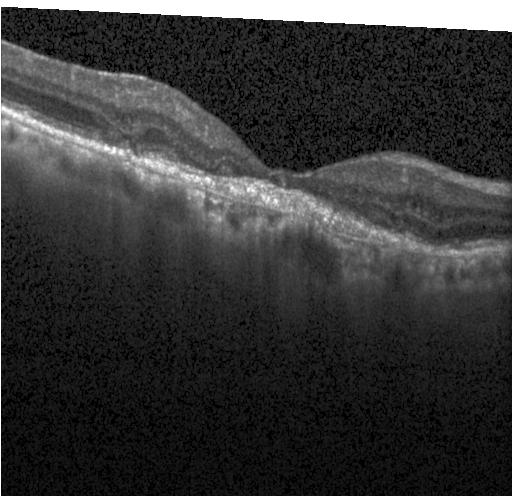 Acquired on a Heidelberg Spectralis, optical coherence tomography B-scan. Diagnosis: choroidal neovascularization.